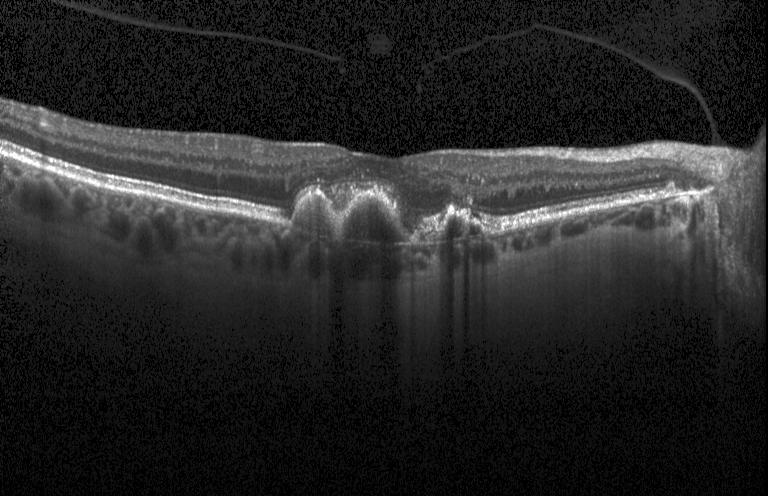
Horizontal scan through the fovea, Heidelberg Spectralis, OCT B-scan, spectral-domain optical coherence tomography. A choroidal neovascular membrane.